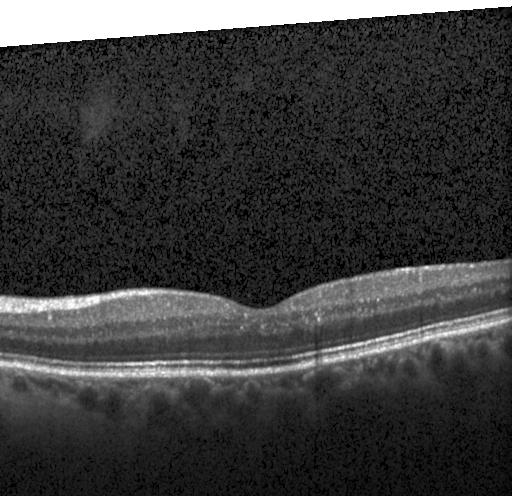 OCT scan showing no evidence of CNV, DME, or drusen.